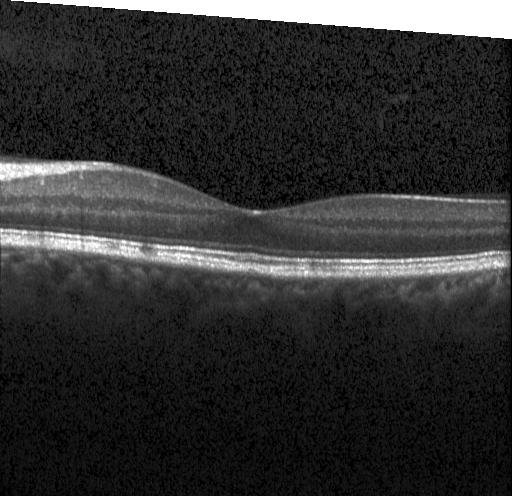

Retinal OCT B-scan
Dx: no choroidal neovascularization, diabetic macular edema, or drusen.